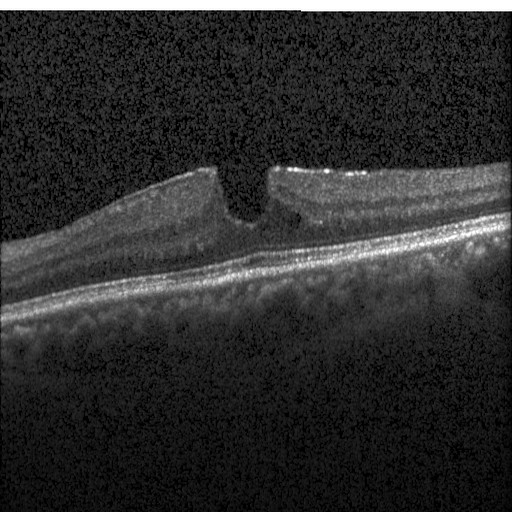 Macular scan · retinal OCT B-scan — The scan shows diabetic macular edema (DME).